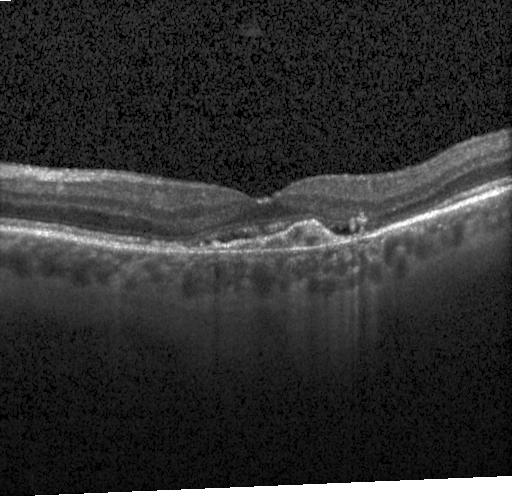 OCT B-scan — Finding: a choroidal neovascular membrane.